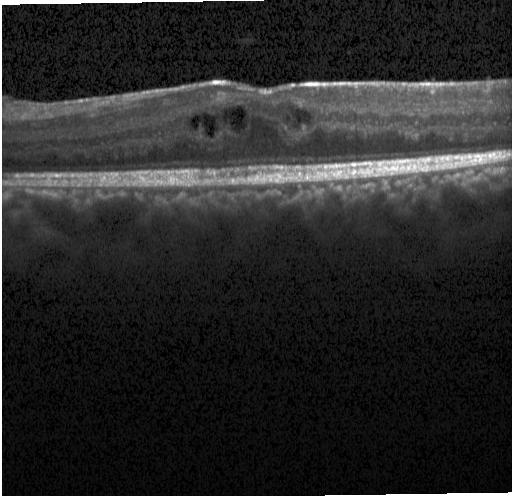

Finding: diabetic macular edema (DME).